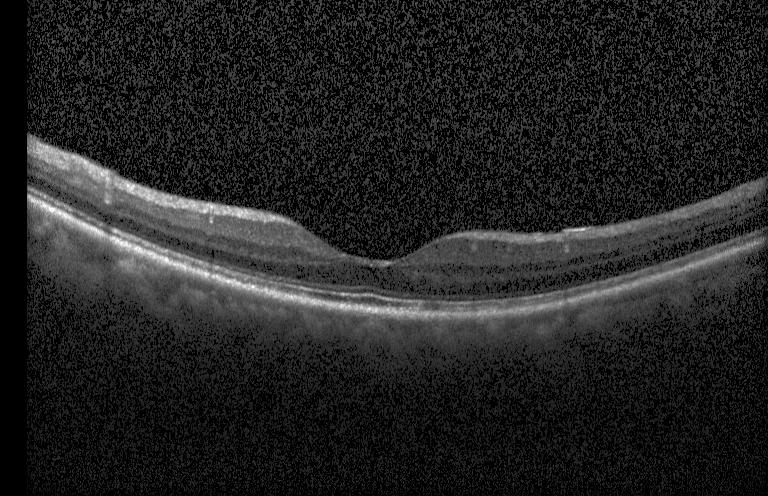 Optical coherence tomography B-scan. Finding: no CNV, no DME, and no drusen.